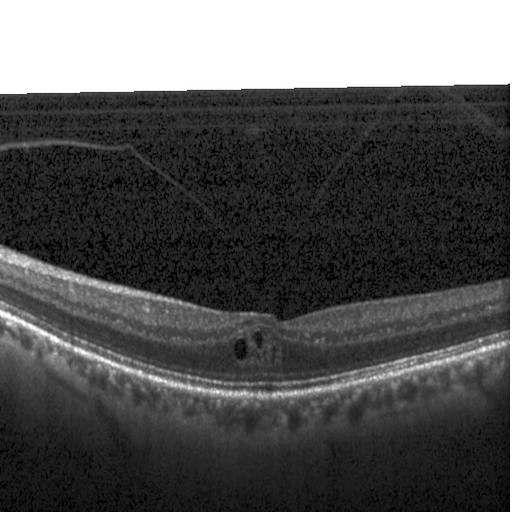 Retinal OCT B-scan · macular scan · SD-OCT · instrument: Heidelberg Spectralis
Finding: diabetic macular edema.